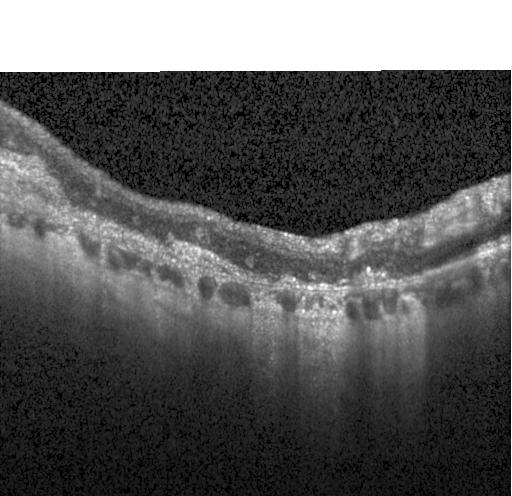

Retinal OCT B-scan · acquired on a Heidelberg Spectralis
A choroidal neovascular membrane.